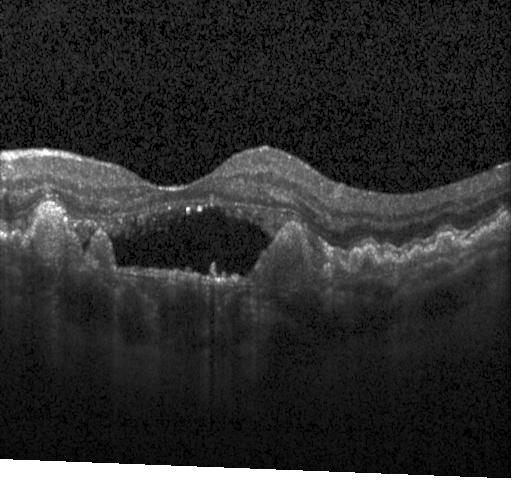 Assessment: a choroidal neovascular membrane.